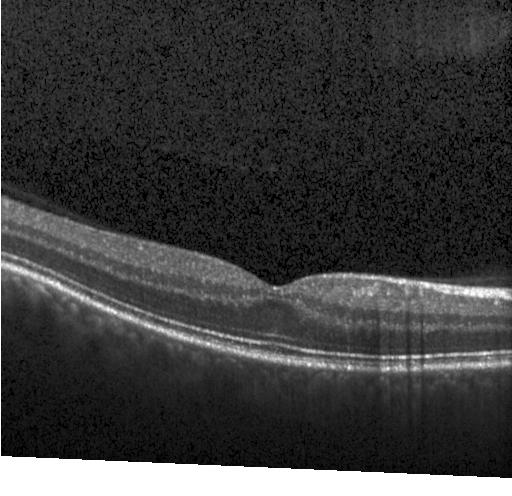
This B-scan demonstrates no evidence of choroidal neovascularization, diabetic macular edema, or drusen.